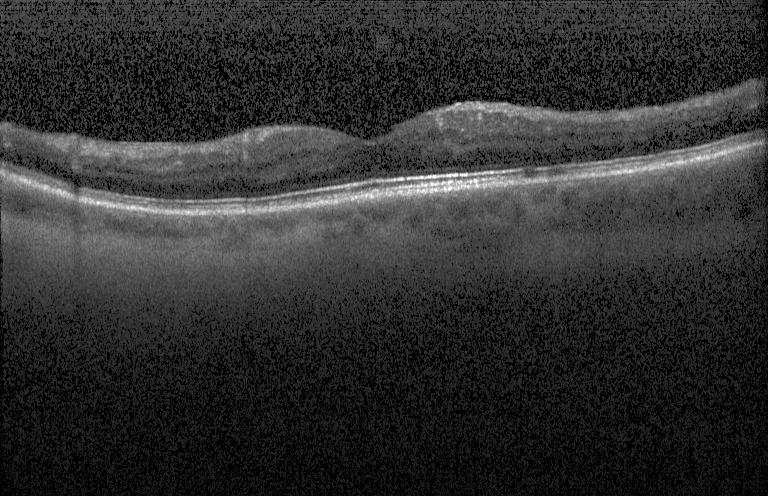 Finding: no CNV, DME, or drusen.